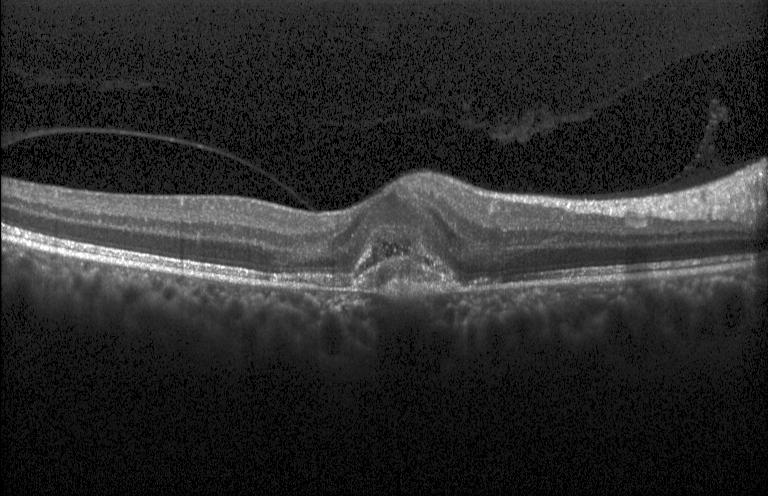
Heidelberg Spectralis · macular scan · retinal OCT cross-section
Impression: a choroidal neovascular membrane.